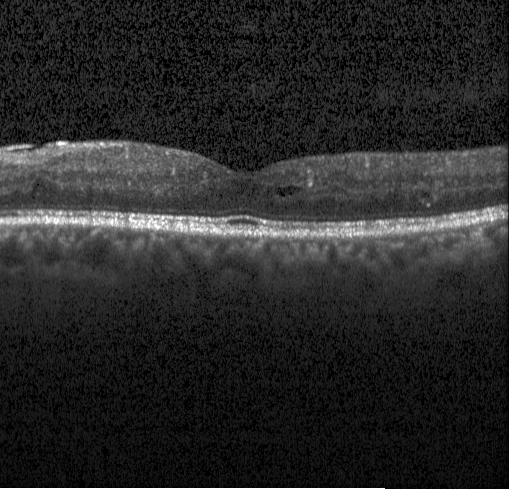 Dx: diabetic macular edema (DME).